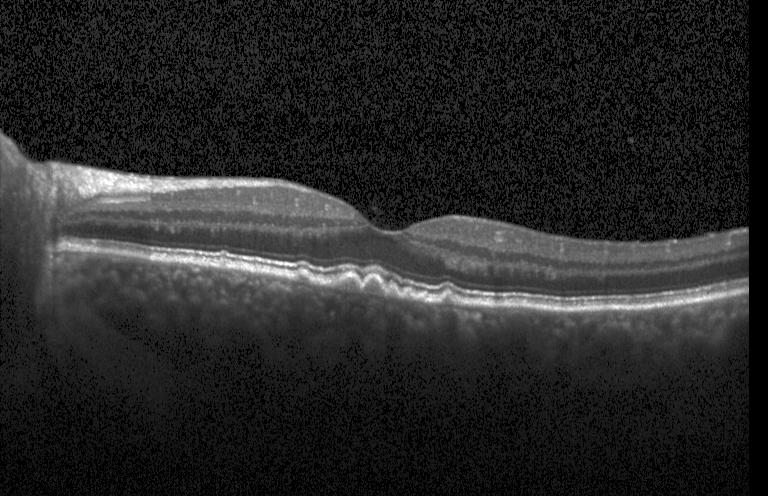

Spectral-domain OCT. OCT line scan.
OCT finding: multiple drusen.